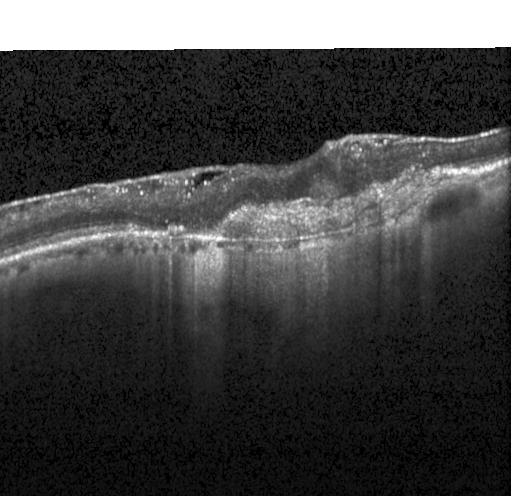 Finding: a choroidal neovascular membrane.